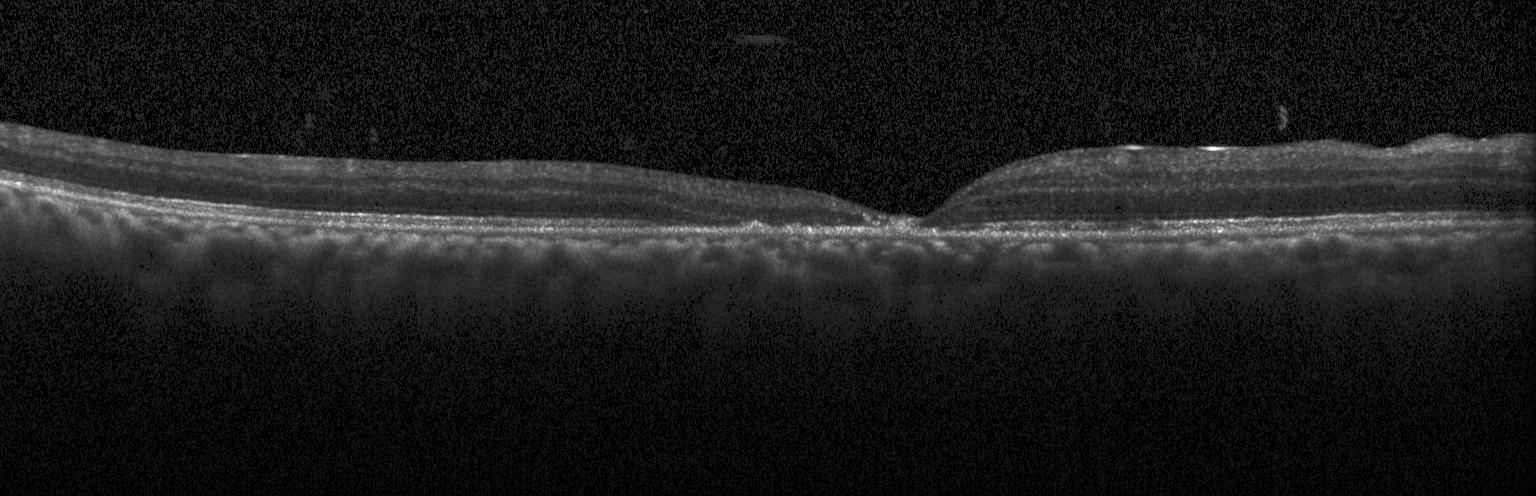 Heidelberg Spectralis OCT system, OCT line scan, macular scan. Diagnosis: no choroidal neovascularization, no diabetic macular edema, and no drusen.